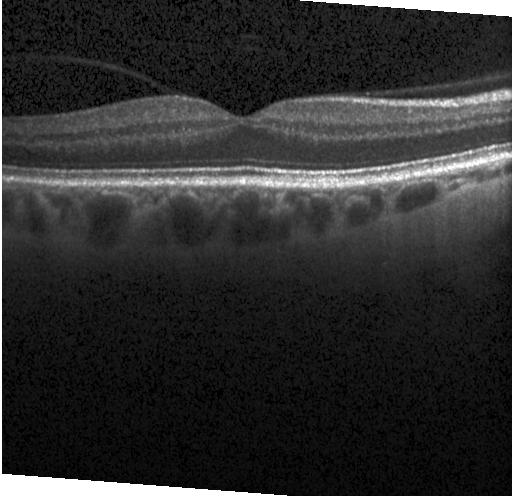

Spectral-domain OCT. Retinal OCT cross-section — Macular OCT: no choroidal neovascularization, no diabetic macular edema, and no drusen.